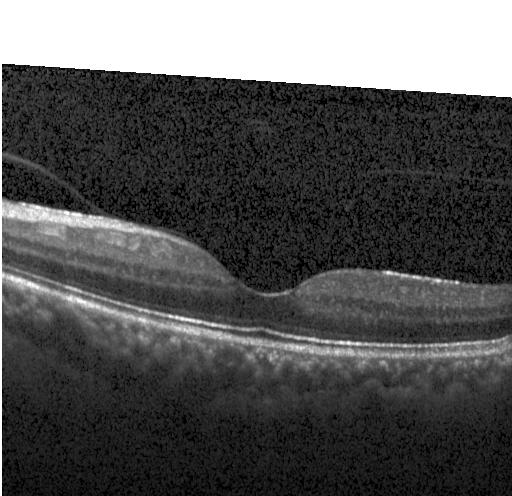
No evidence of CNV, DME, or drusen.